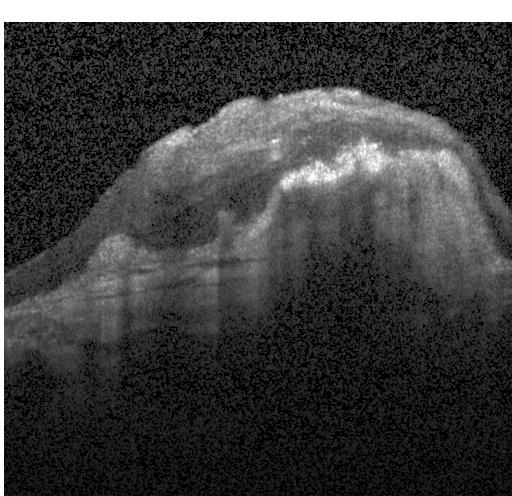
Finding: a choroidal neovascular membrane.